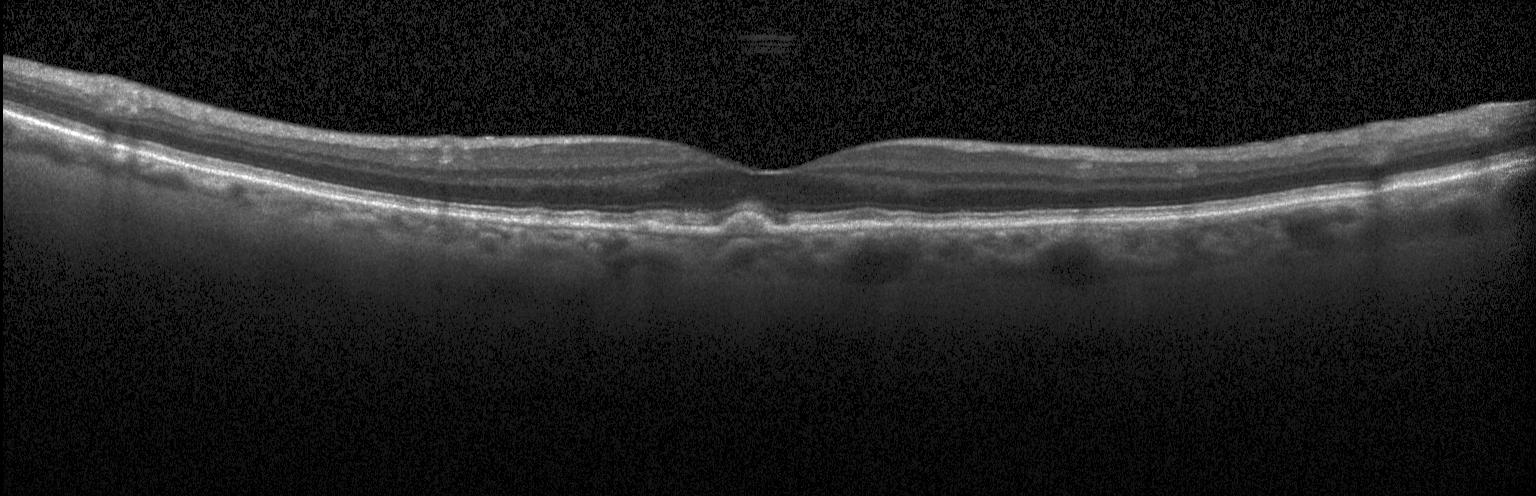 The scan shows sub-RPE drusenoid deposits.